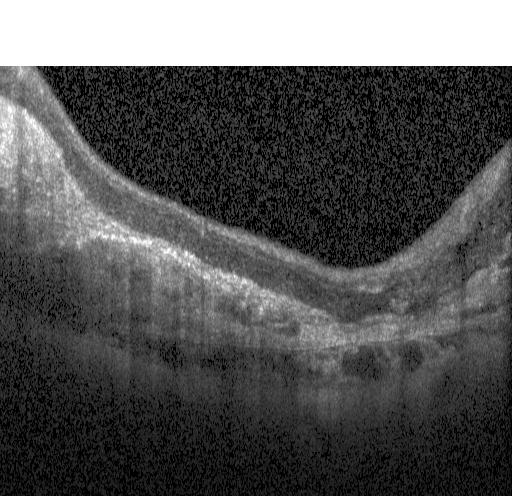 Dx: choroidal neovascularization.